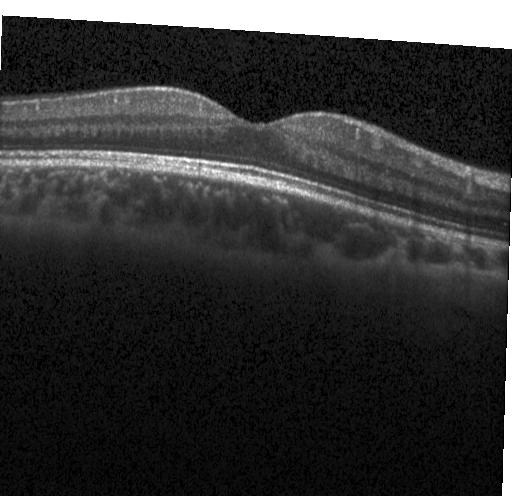

Retinal OCT B-scan. Macular OCT: no CNV, DME, or drusen.